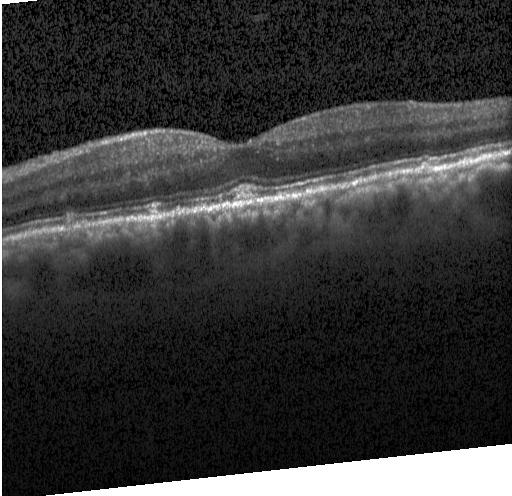 Fovea-centered; OCT B-scan.
Diagnosis: sub-RPE drusenoid deposits.